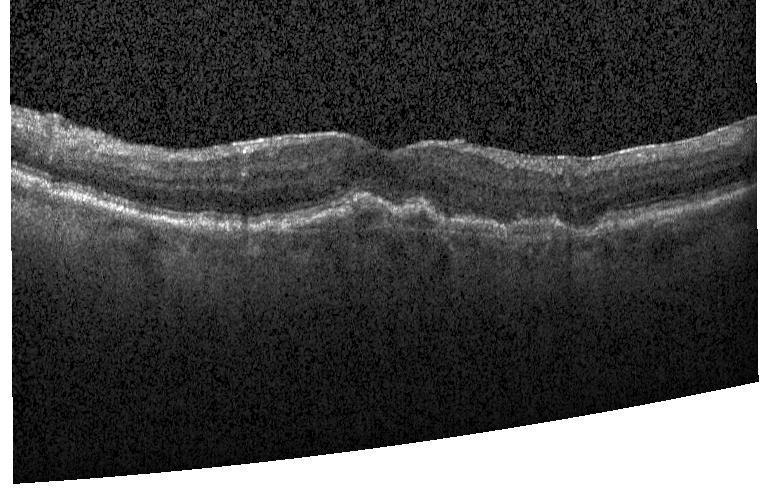
OCT B-scan, spectral-domain optical coherence tomography, fovea-centered, Heidelberg Spectralis — OCT finding: a choroidal neovascular membrane.